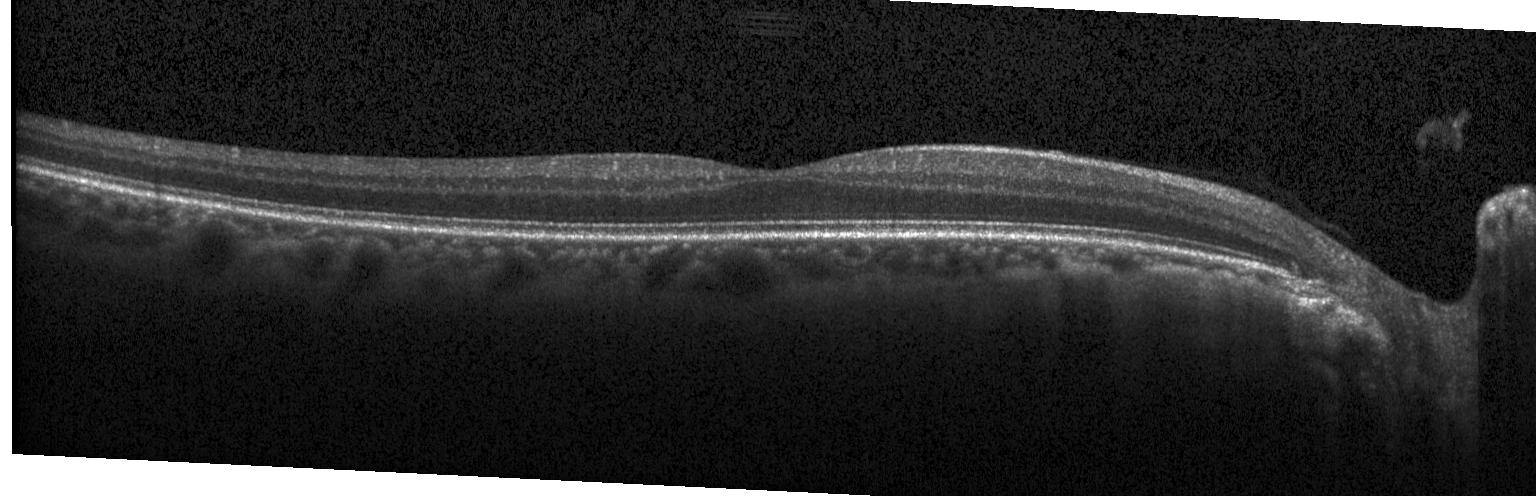 This B-scan demonstrates neither CNV, DME, nor drusen.